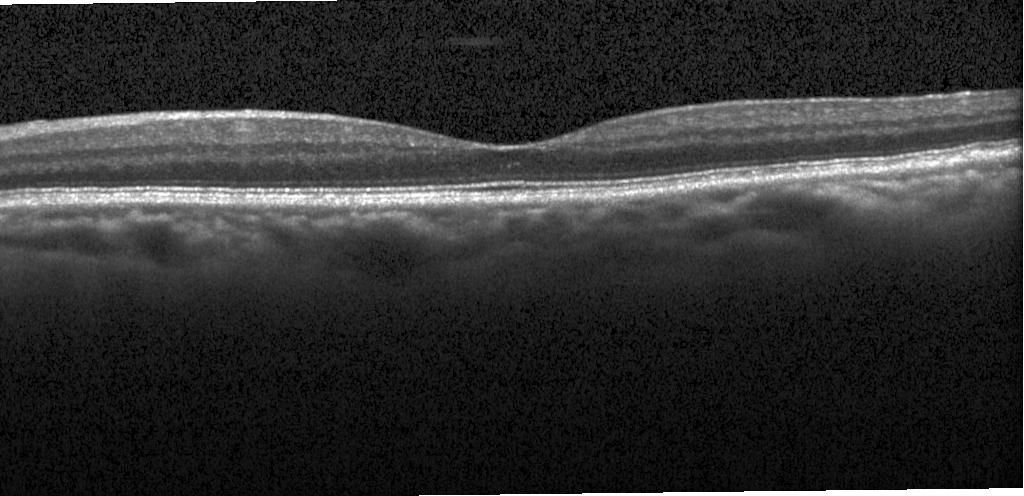
Optical coherence tomography B-scan — Assessment: neither choroidal neovascularization, diabetic macular edema, nor drusen.